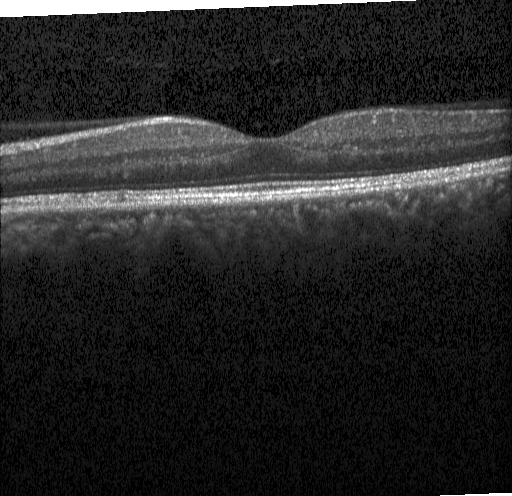 Retinal OCT cross-section showing neither choroidal neovascularization, diabetic macular edema, nor drusen.